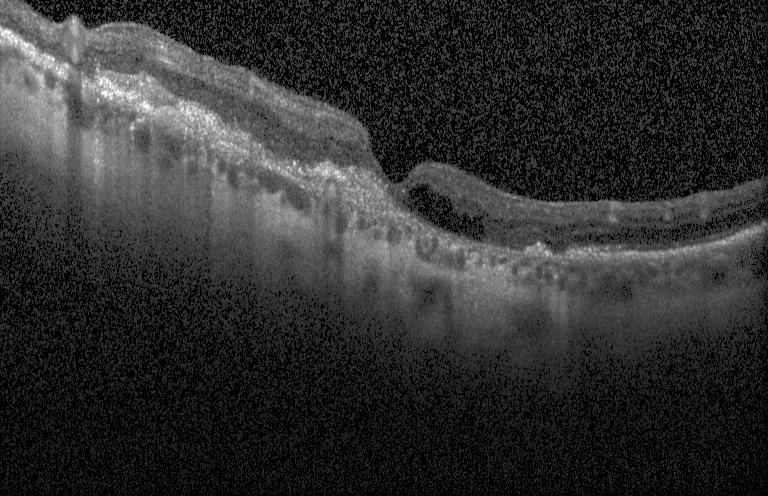

Instrument: Heidelberg Spectralis · optical coherence tomography B-scan.
Diagnosis: a choroidal neovascular membrane.